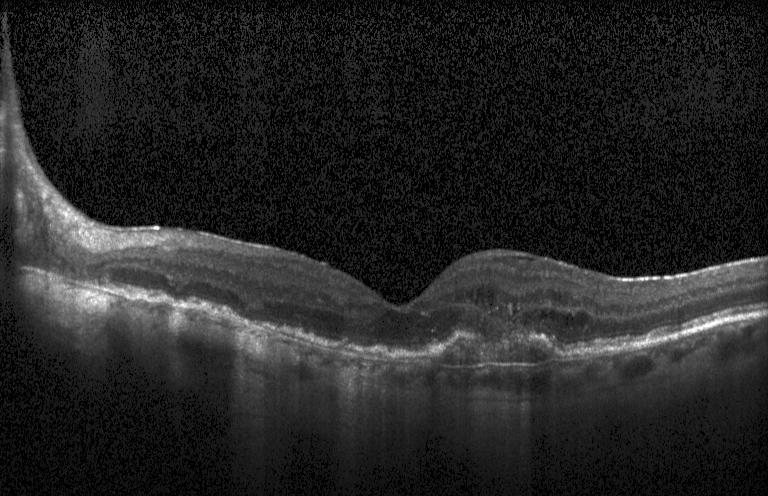 Macular OCT: a choroidal neovascular membrane.